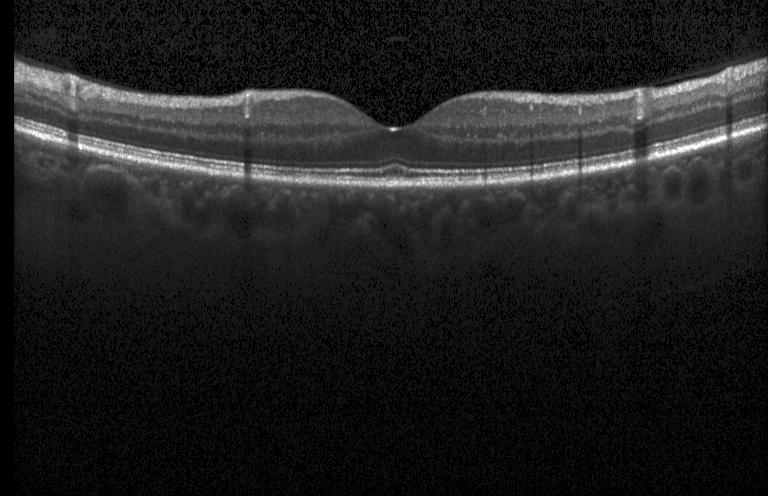

Acquired on a Heidelberg Spectralis, retinal OCT cross-section, centered on the fovea. This B-scan demonstrates no choroidal neovascularization, diabetic macular edema, or drusen.